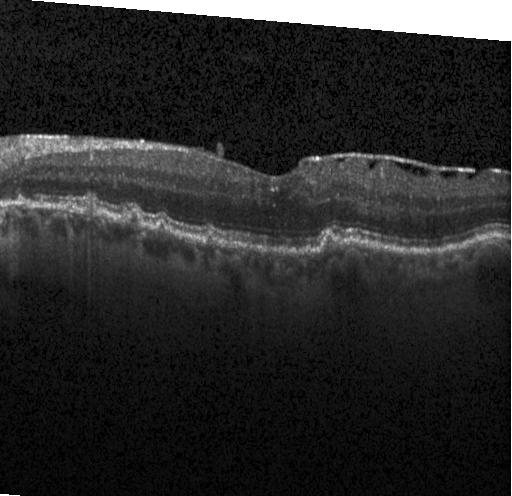
Retinal OCT B-scan
Drusen.